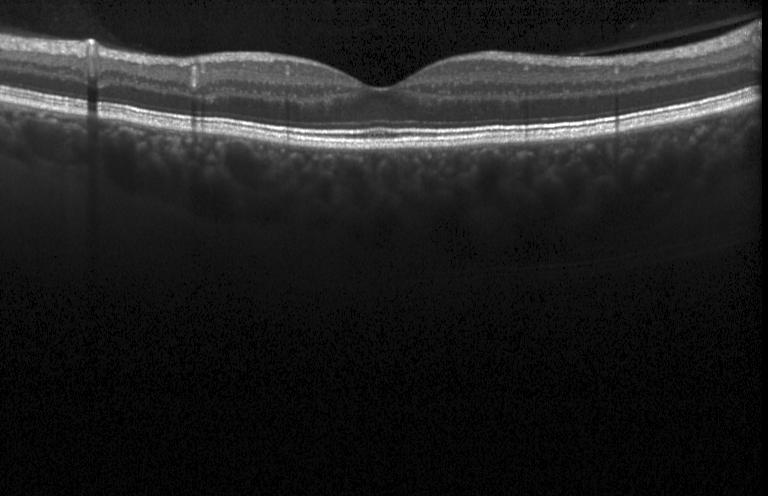
Retinal OCT B-scan
This B-scan demonstrates neither choroidal neovascularization, diabetic macular edema, nor drusen.